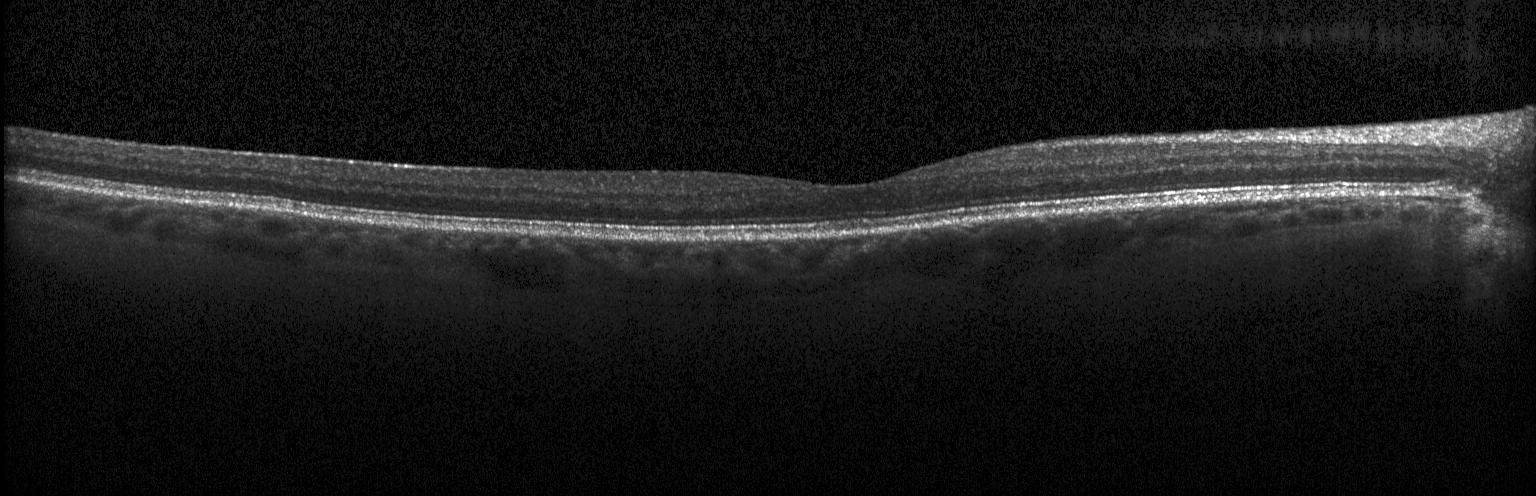

Macular OCT: no choroidal neovascularization, diabetic macular edema, or drusen.